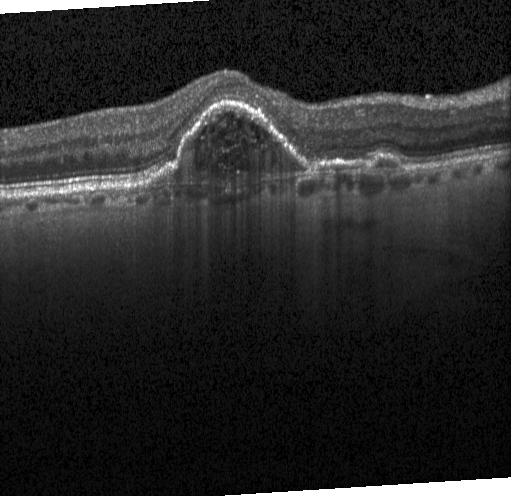 Retinal OCT B-scan. Heidelberg Spectralis OCT system. Fovea-centered — Diagnosis: choroidal neovascularization (CNV).